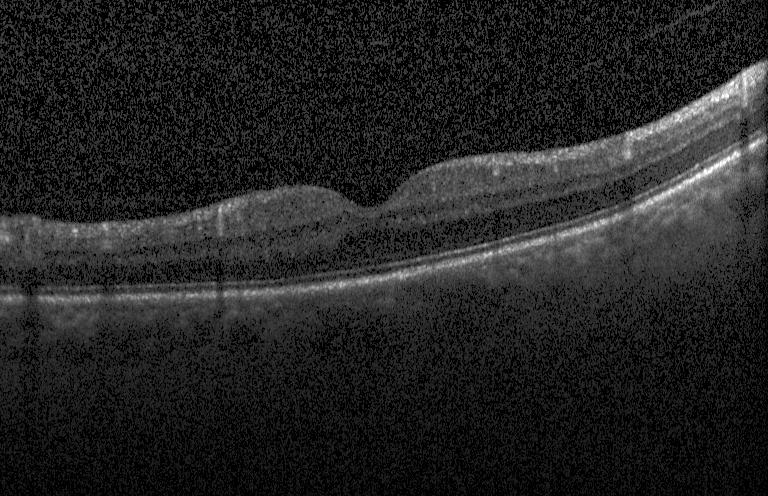
SD-OCT · retinal OCT B-scan · centered on the fovea · acquired on a Heidelberg Spectralis. The scan shows no CNV, DME, or drusen.